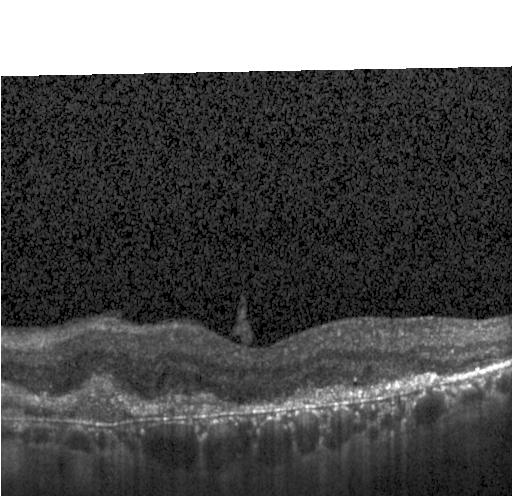

Horizontal scan through the fovea; optical coherence tomography B-scan; spectral-domain optical coherence tomography; instrument: Heidelberg Spectralis
Dx: a choroidal neovascular membrane.